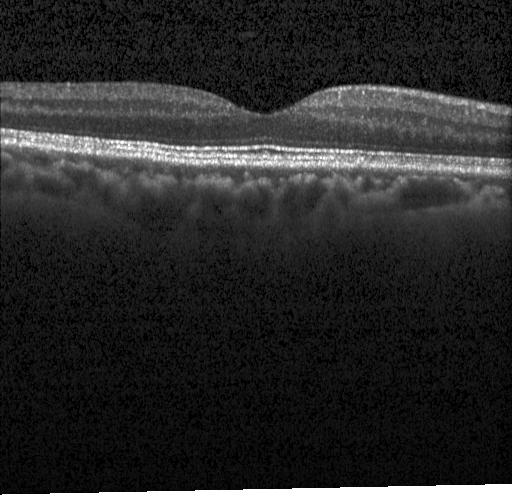 Centered on the fovea. Optical coherence tomography scan. SD-OCT — Diagnosis: no CNV, no DME, and no drusen.